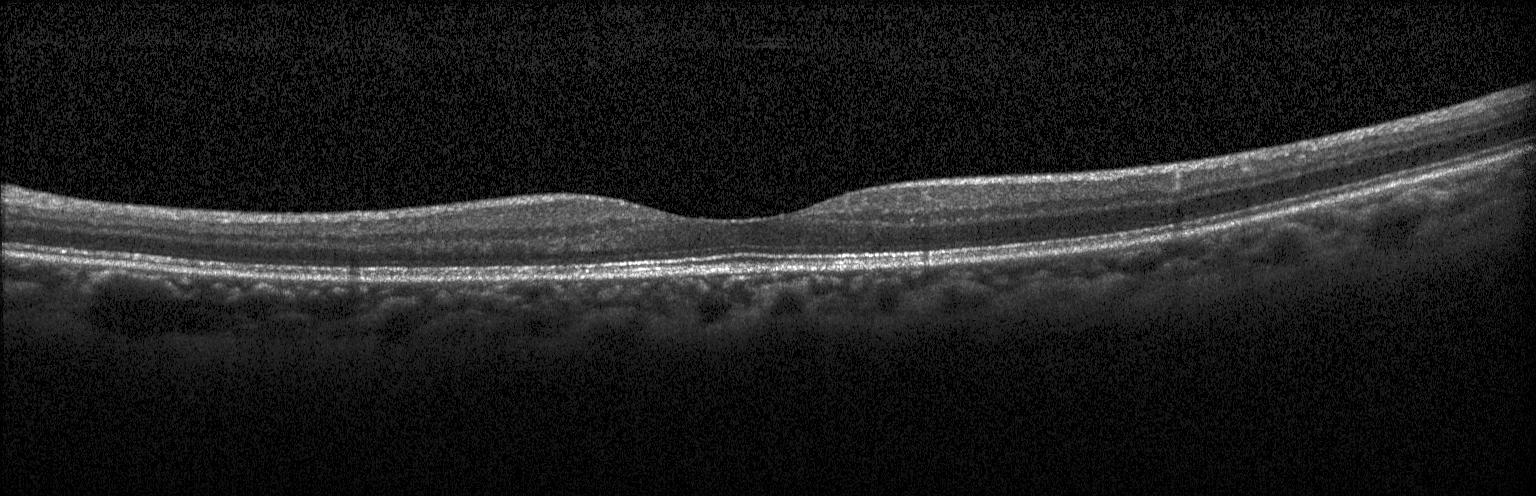

OCT B-scan. Centered on the fovea
Impression: no choroidal neovascularization, no diabetic macular edema, and no drusen.